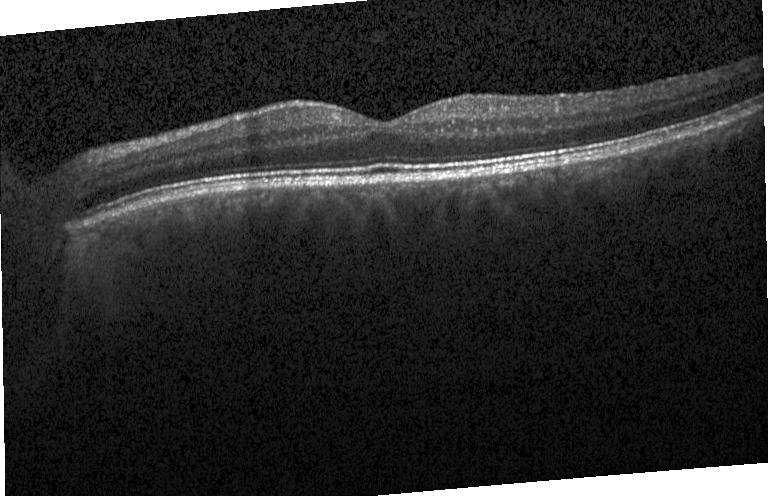
Optical coherence tomography B-scan · spectral-domain OCT. Diagnosis: no CNV, no DME, and no drusen.